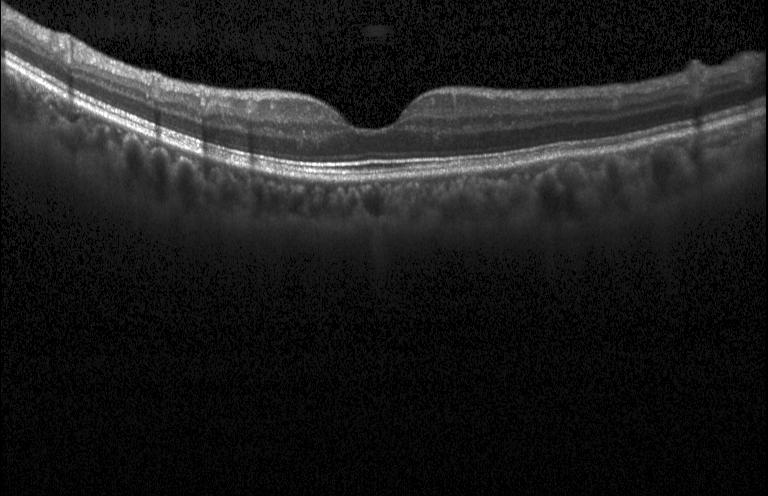
Assessment: neither CNV, DME, nor drusen.